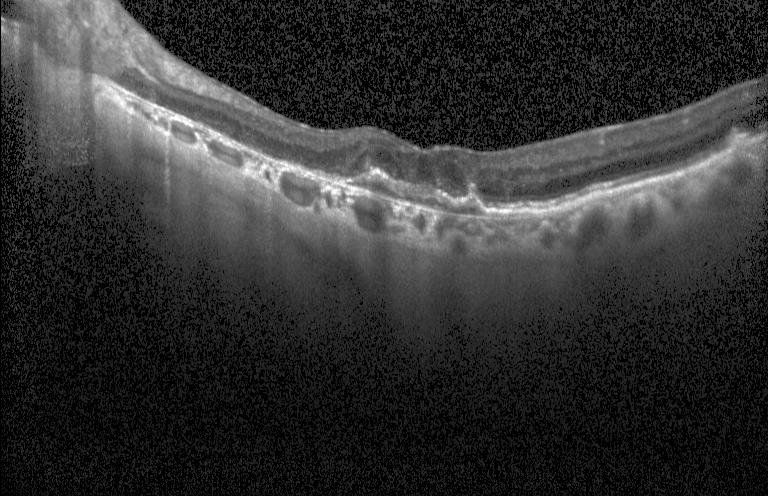 Retinal OCT cross-section. Finding: CNV.